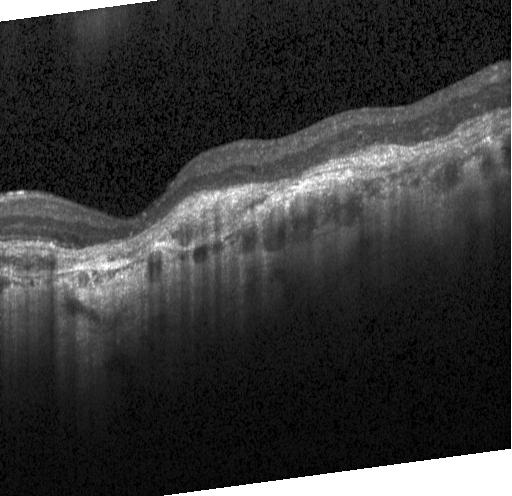
Macular OCT: choroidal neovascularization.